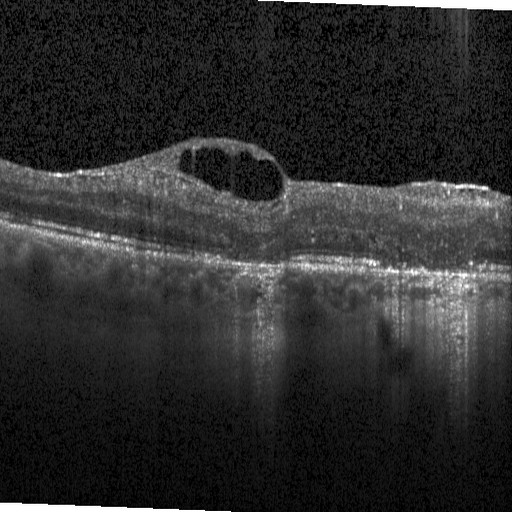
Heidelberg Spectralis; SD-OCT; OCT line scan. Macular OCT: DME.